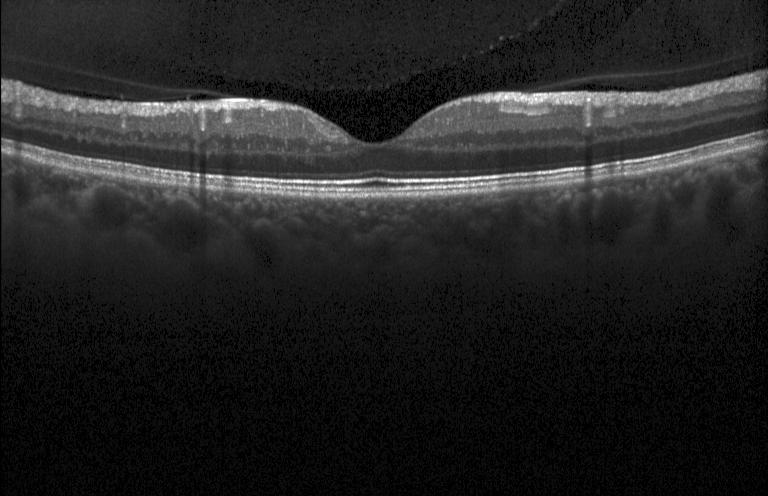
SD-OCT. Heidelberg Spectralis. Retinal OCT B-scan. Centered on the fovea.
Macular OCT: no evidence of choroidal neovascularization, diabetic macular edema, or drusen.